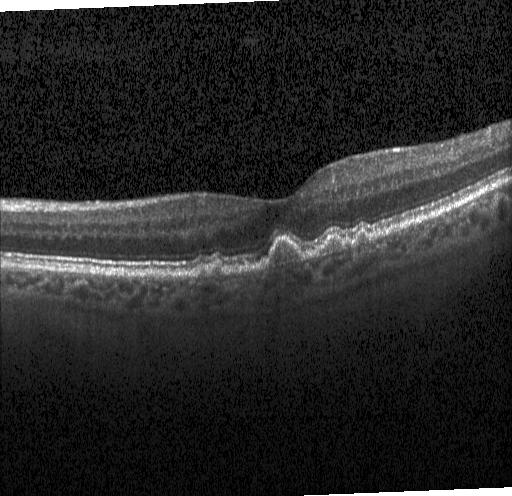
Retinal OCT cross-section showing sub-RPE drusenoid deposits.